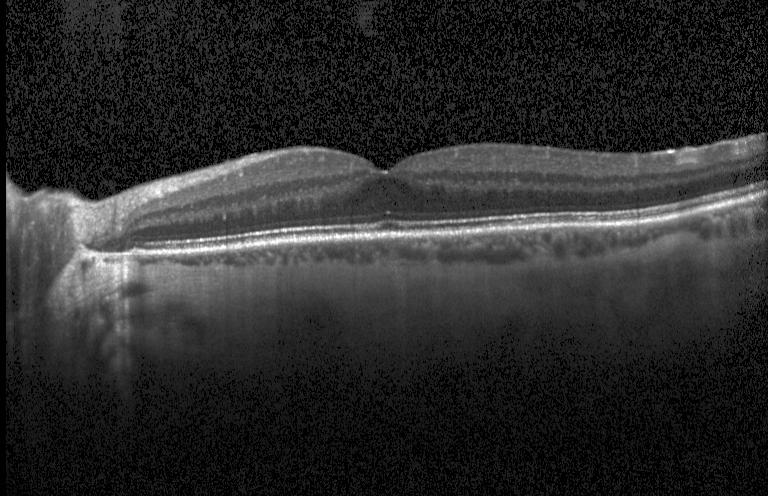 Spectral-domain optical coherence tomography, Heidelberg Spectralis OCT system, OCT B-scan — Assessment: no evidence of choroidal neovascularization, diabetic macular edema, or drusen.